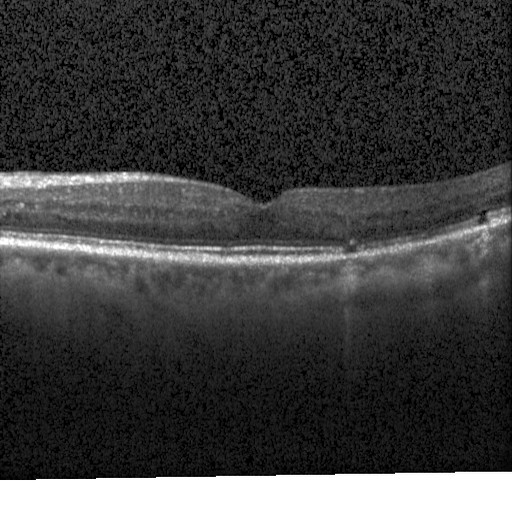

Optical coherence tomography scan. Heidelberg Spectralis.
Finding: diabetic macular edema.